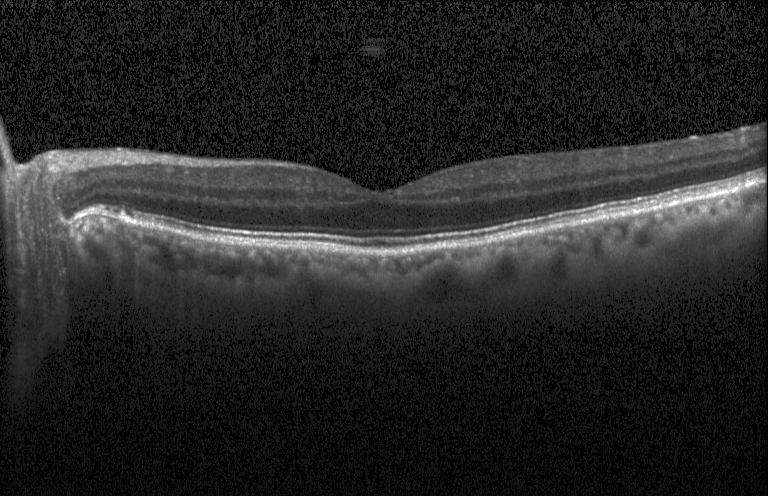

Finding: no choroidal neovascularization, diabetic macular edema, or drusen.